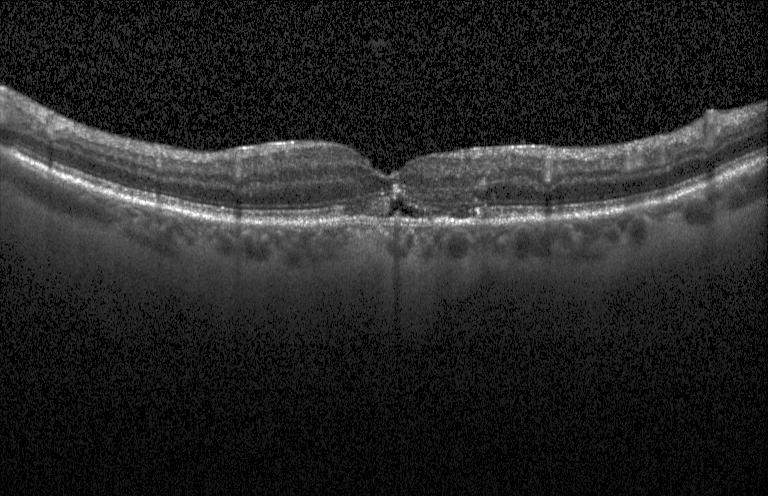

Retinal OCT cross-section. SD-OCT. Heidelberg Spectralis OCT system
Assessment: a choroidal neovascular membrane.